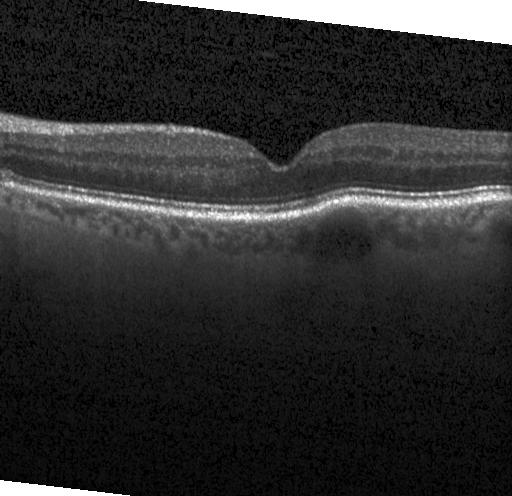
Instrument: Heidelberg Spectralis · optical coherence tomography scan · SD-OCT. Finding: no evidence of choroidal neovascularization, diabetic macular edema, or drusen.